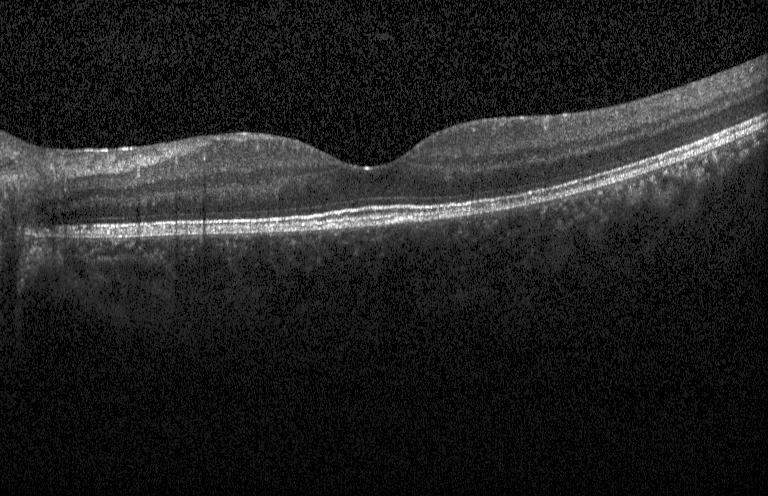 Heidelberg Spectralis OCT system; optical coherence tomography B-scan. Finding: neither CNV, DME, nor drusen.